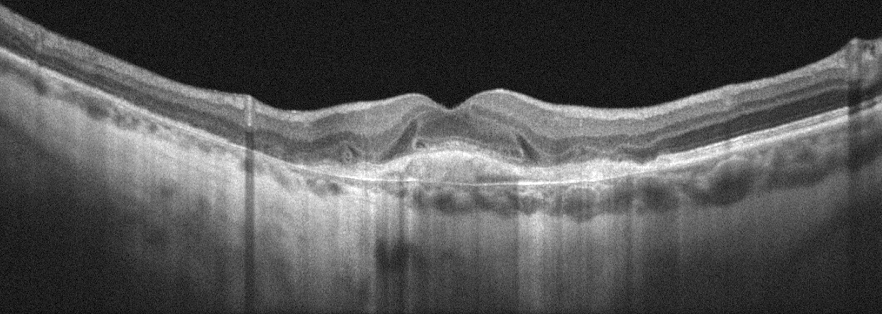 Optovue Avanti RTVue XR; OD; optical coherence tomography scan.
Impression: age-related macular degeneration (AMD).